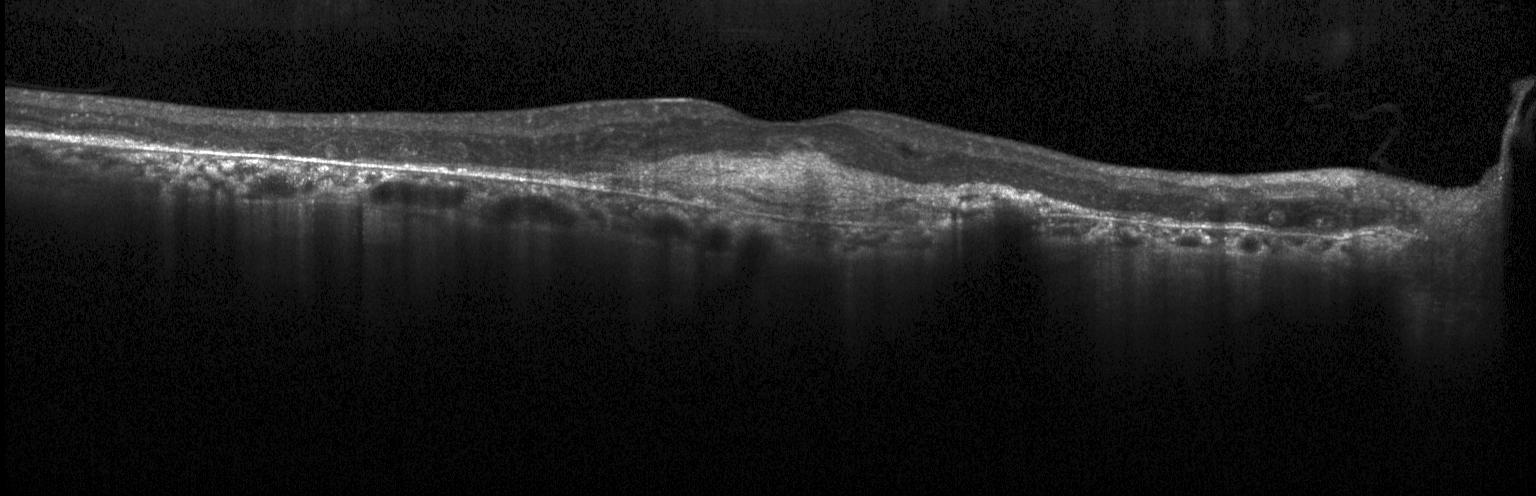 OCT B-scan — The scan shows a choroidal neovascular membrane.